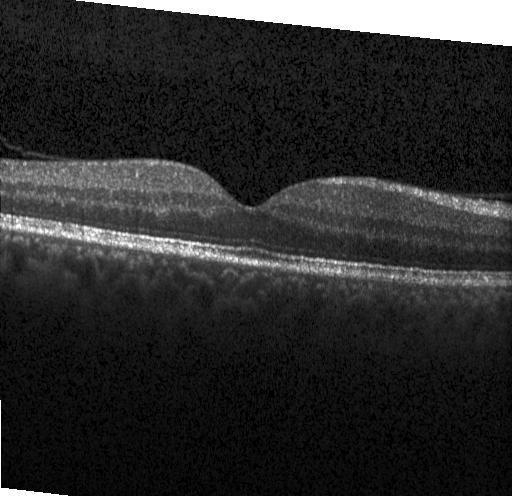

Optical coherence tomography scan. Spectral-domain optical coherence tomography
Finding: no evidence of choroidal neovascularization, diabetic macular edema, or drusen.